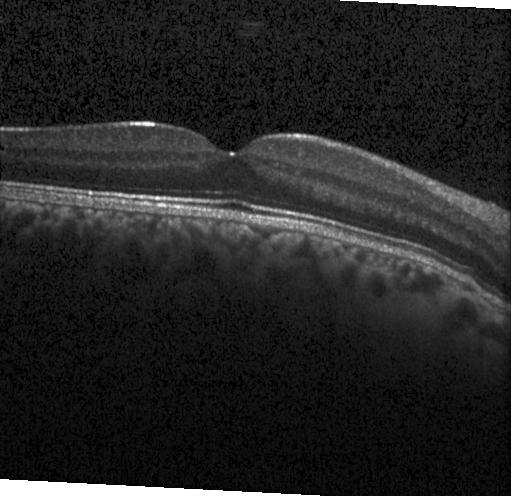

The scan shows no choroidal neovascularization, no diabetic macular edema, and no drusen.